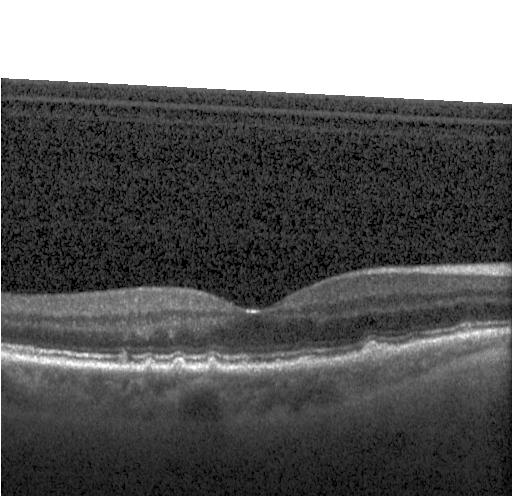

Optical coherence tomography B-scan; spectral-domain optical coherence tomography
Assessment: drusen.